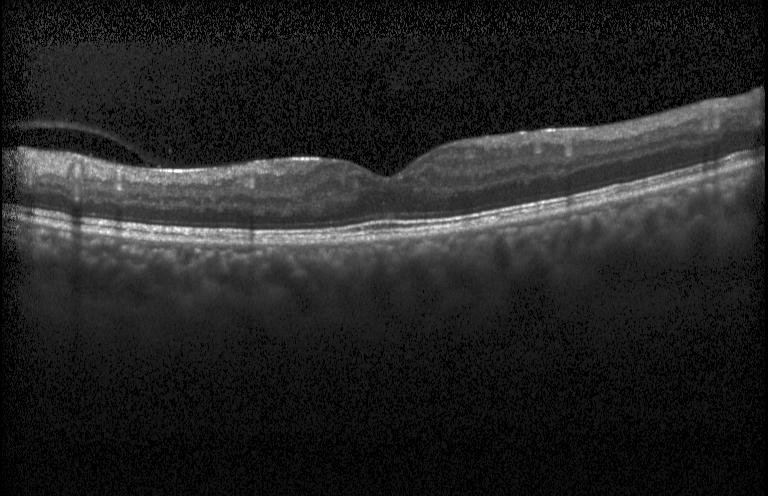 Retinal OCT B-scan · macular scan — Finding: no choroidal neovascularization, diabetic macular edema, or drusen.